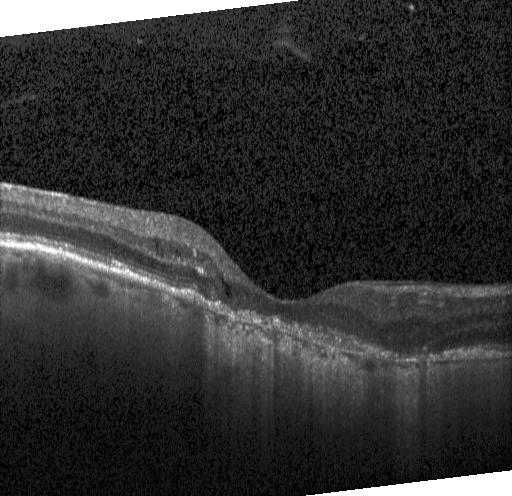 Fovea-centered, optical coherence tomography B-scan, instrument: Heidelberg Spectralis, spectral-domain OCT.
Finding: choroidal neovascularization.